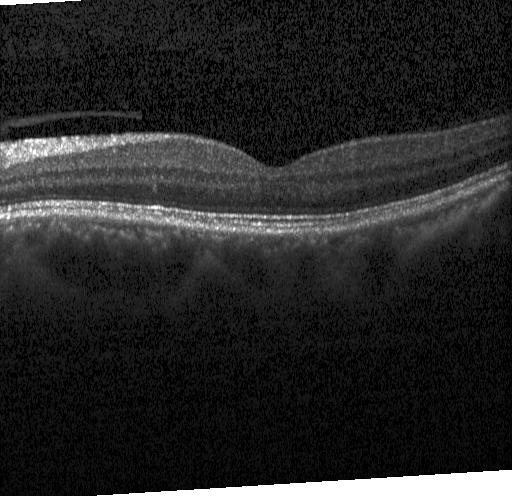

Heidelberg Spectralis OCT system. OCT B-scan — Diagnosis: no evidence of choroidal neovascularization, diabetic macular edema, or drusen.